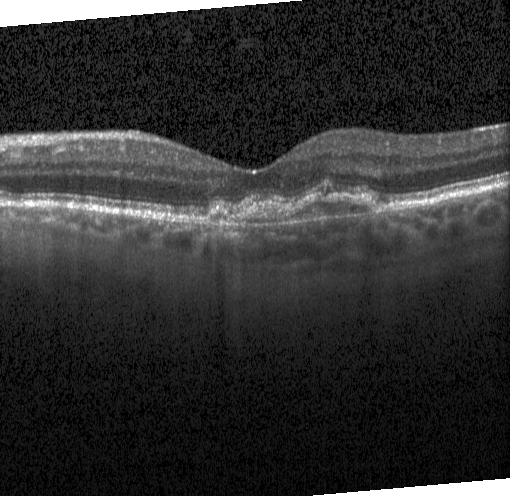 Macular OCT: a choroidal neovascular membrane.